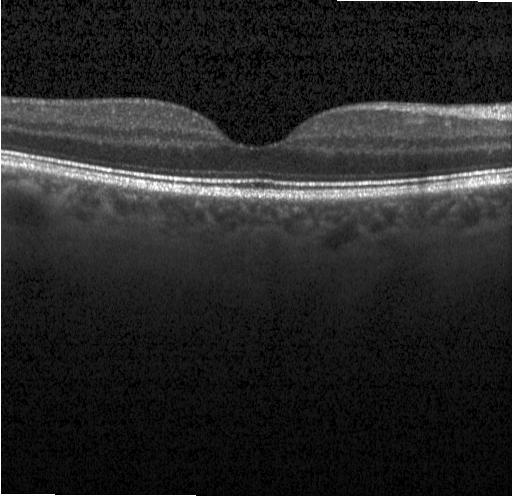
Optical coherence tomography scan.
Diagnosis: no evidence of CNV, DME, or drusen.